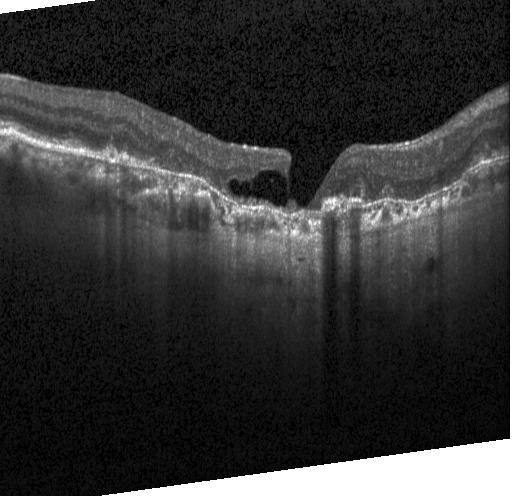
OCT finding: a choroidal neovascular membrane.